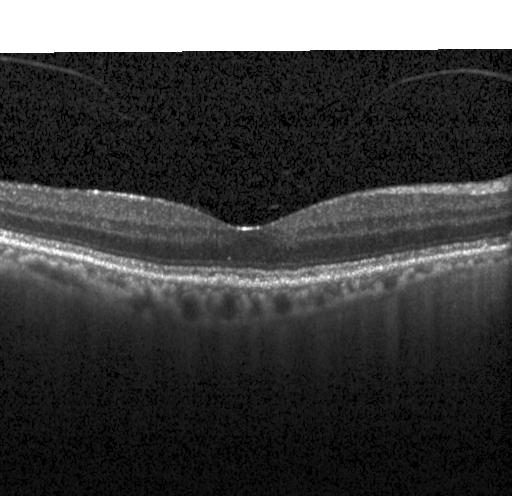

Retinal OCT cross-section, fovea-centered
Finding: no evidence of CNV, DME, or drusen.